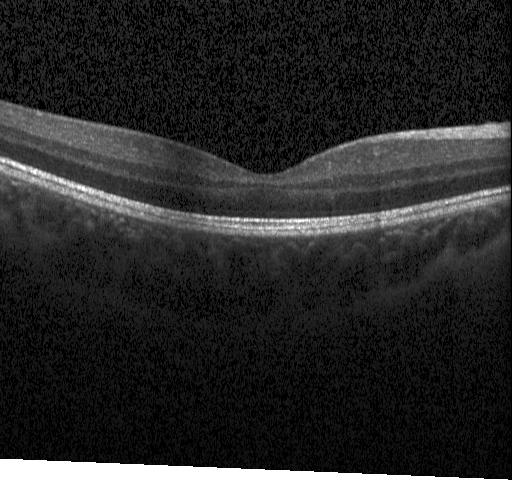

Spectral-domain OCT B-scan: neither choroidal neovascularization, diabetic macular edema, nor drusen.